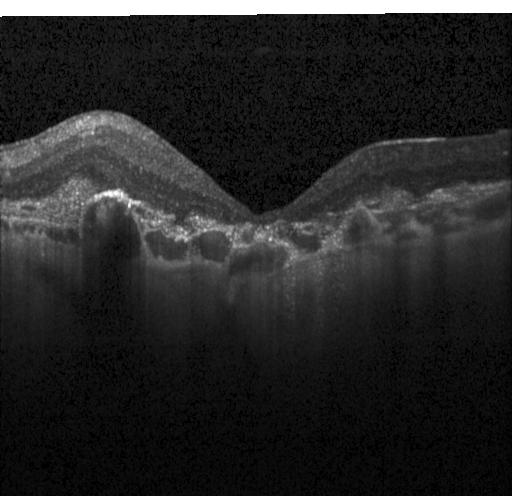 Diagnosis: choroidal neovascularization.